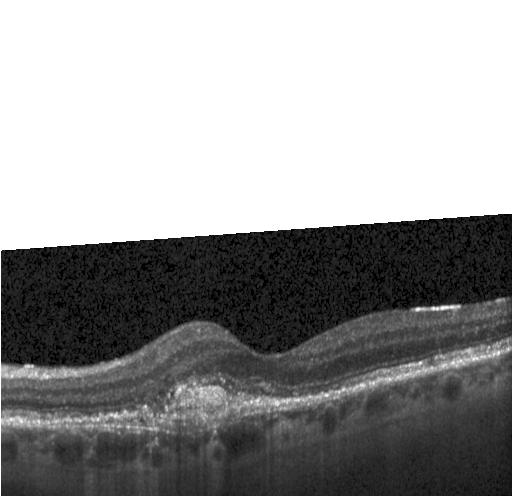

Centered on the fovea. Heidelberg Spectralis OCT system. Optical coherence tomography scan. Spectral-domain OCT.
OCT finding: choroidal neovascularization (CNV).